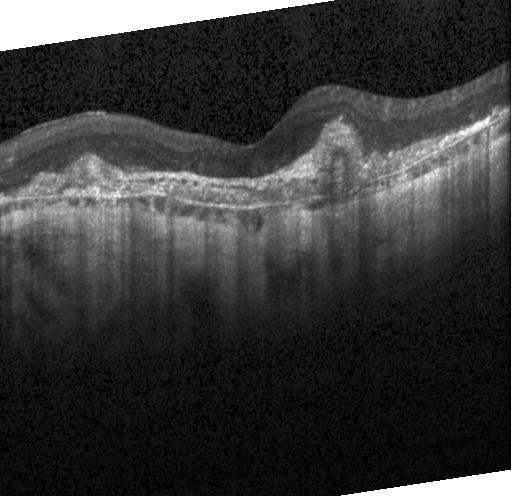 Acquired on a Heidelberg Spectralis, optical coherence tomography scan. OCT finding: a choroidal neovascular membrane.